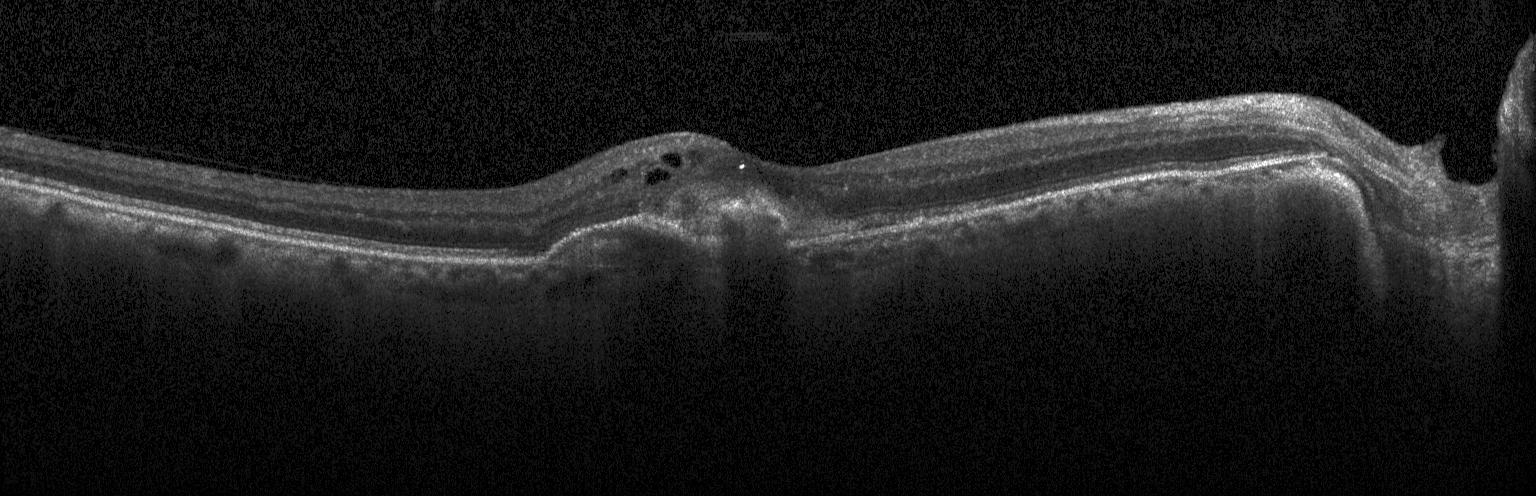
OCT B-scan — Impression: choroidal neovascularization (CNV).